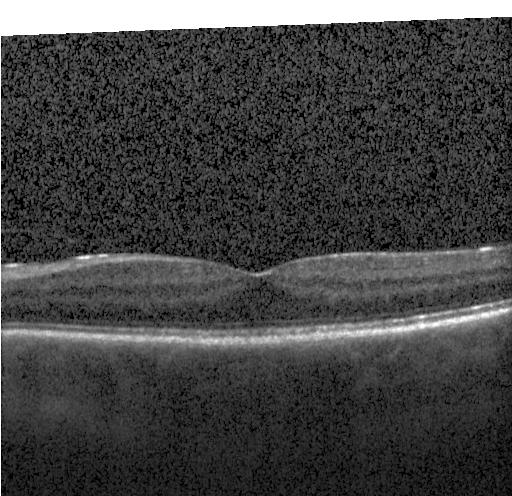

Optical coherence tomography B-scan.
No evidence of choroidal neovascularization, diabetic macular edema, or drusen.